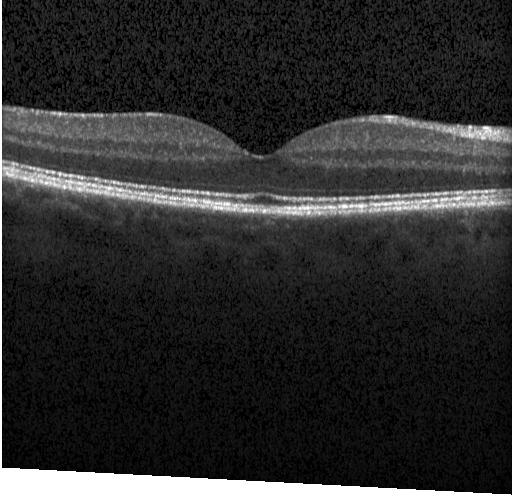 Finding: no CNV, no DME, and no drusen.